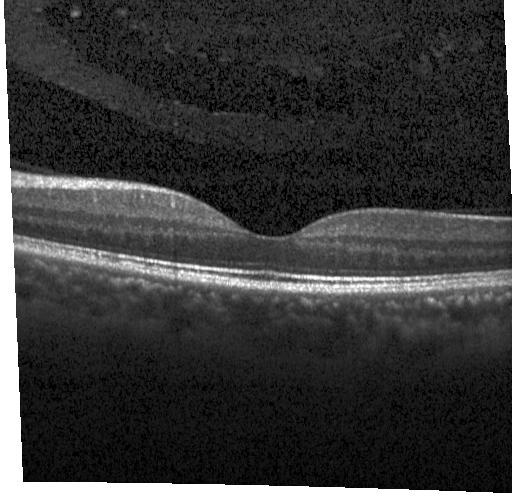 Retinal OCT B-scan
Impression: no evidence of choroidal neovascularization, diabetic macular edema, or drusen.